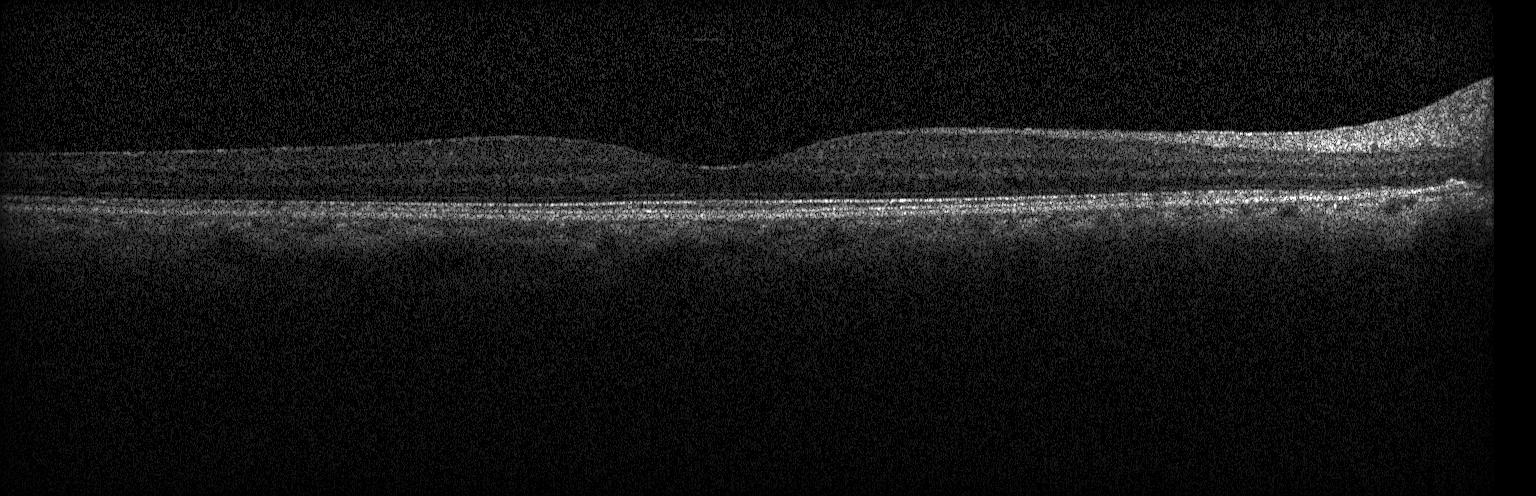

The scan shows no choroidal neovascularization, no diabetic macular edema, and no drusen.